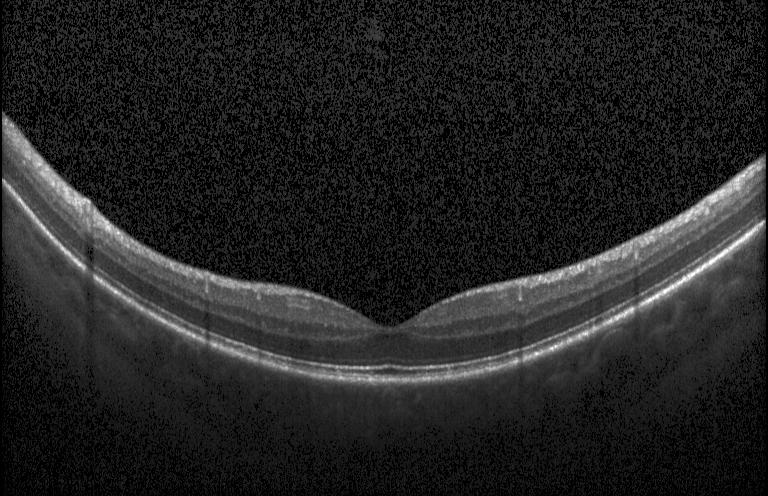
Retinal OCT cross-section showing no CNV, DME, or drusen.